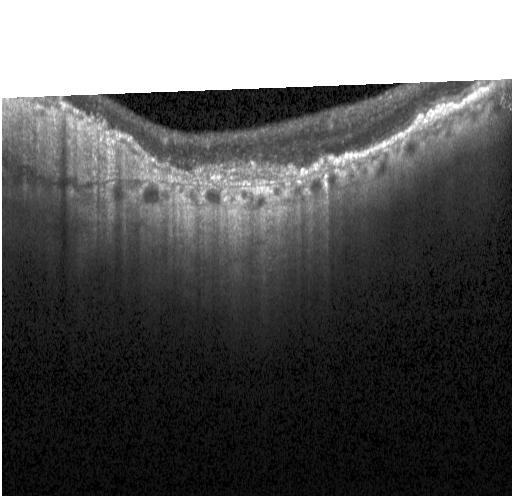

This B-scan demonstrates choroidal neovascularization (CNV).